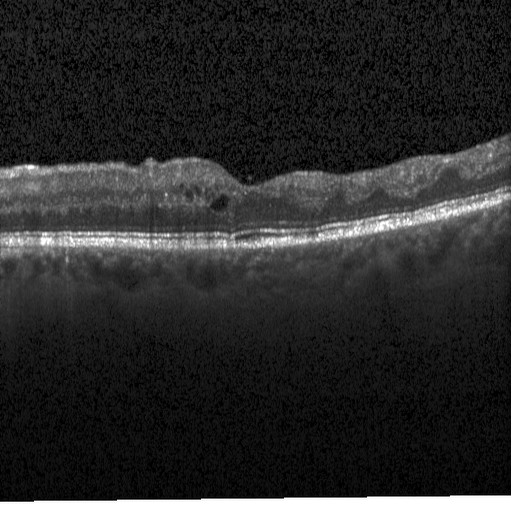 Diagnosis: diabetic macular edema.